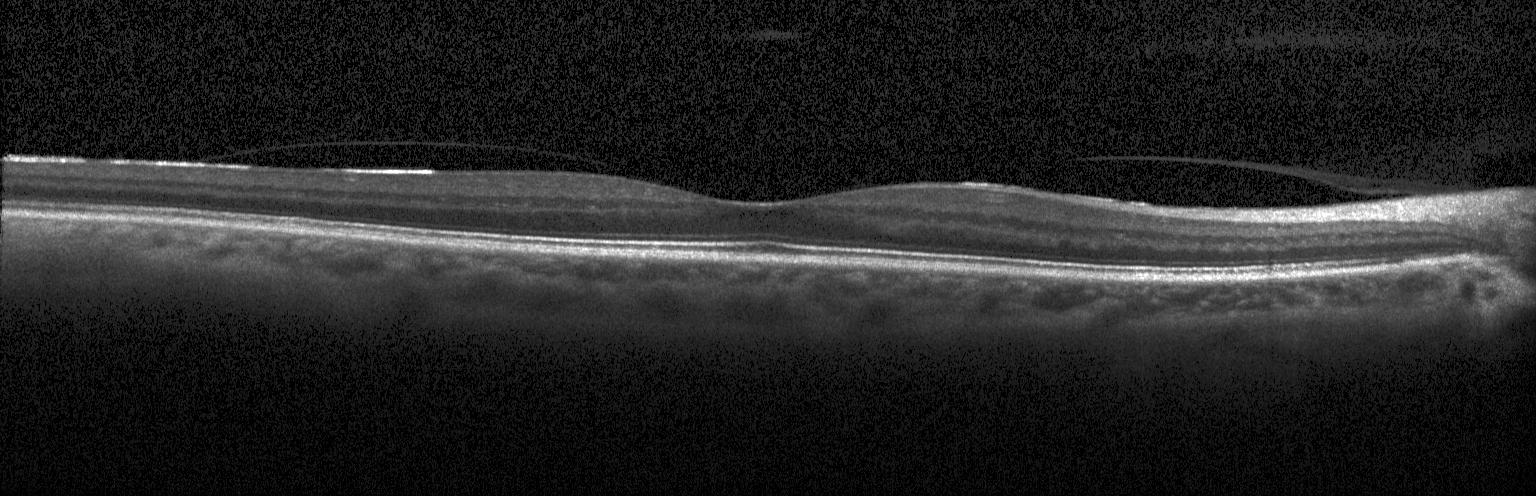 Acquired on a Heidelberg Spectralis; retinal OCT cross-section; horizontal scan through the fovea — Impression: no evidence of choroidal neovascularization, diabetic macular edema, or drusen.